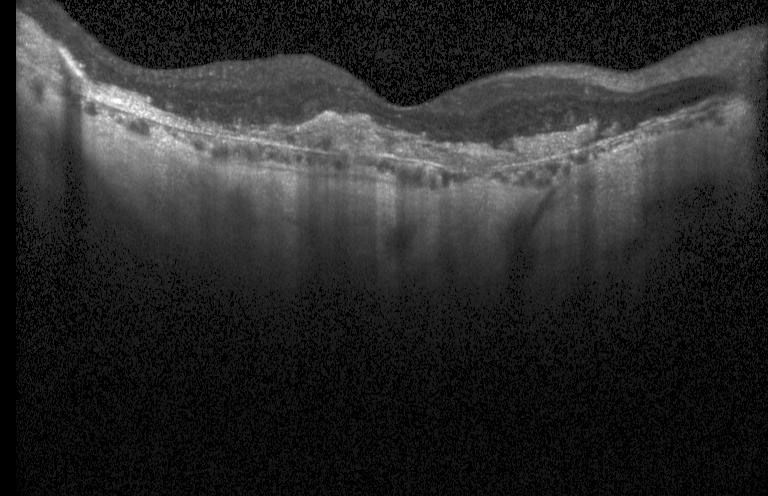
Horizontal scan through the fovea; OCT line scan — Impression: choroidal neovascularization.